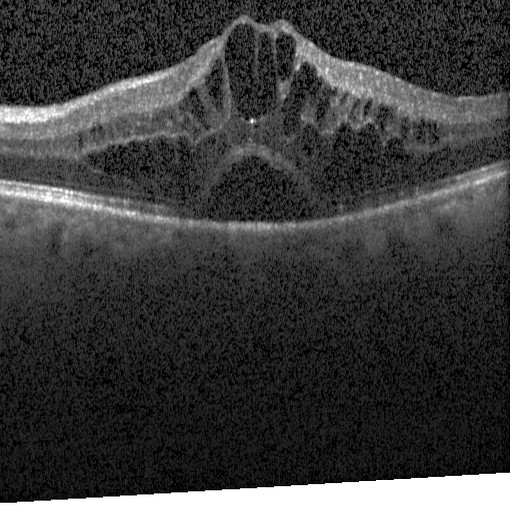
SD-OCT · retinal OCT cross-section
Assessment: diabetic macular edema.